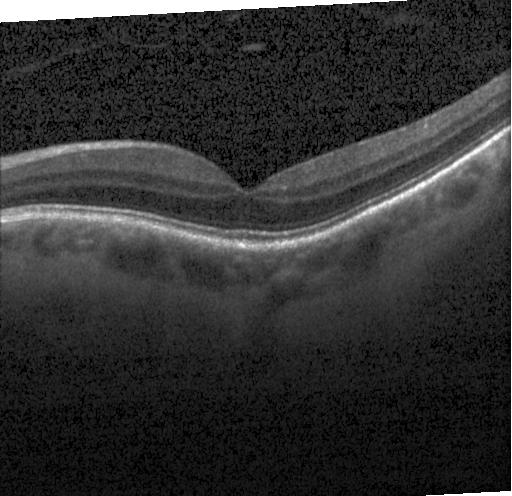
Optical coherence tomography scan · through the macula.
Impression: no CNV, no DME, and no drusen.